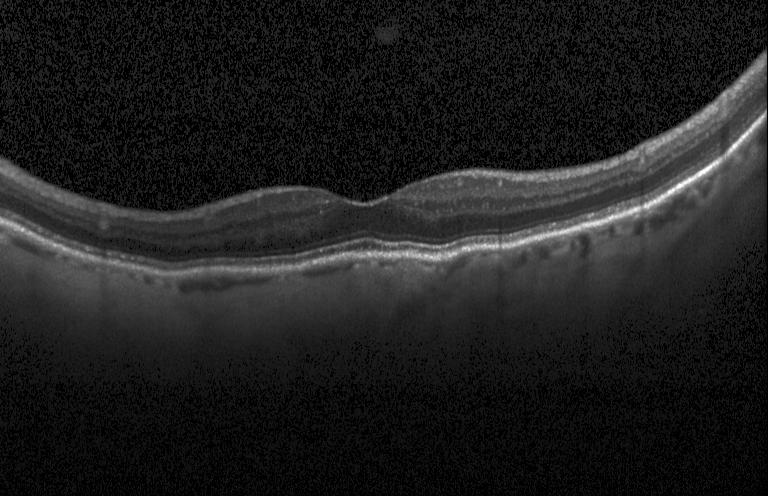
The scan shows no evidence of CNV, DME, or drusen.